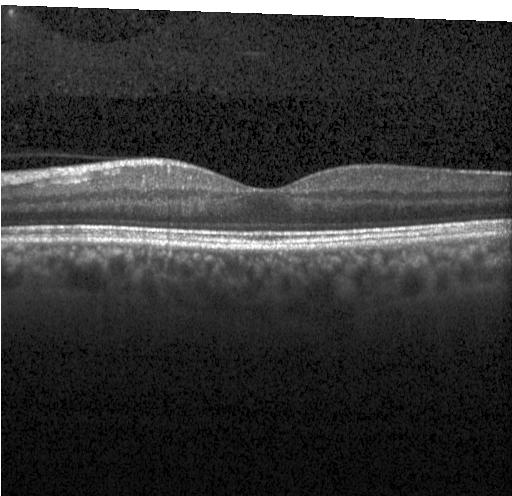

Retinal OCT B-scan — No choroidal neovascularization, no diabetic macular edema, and no drusen.